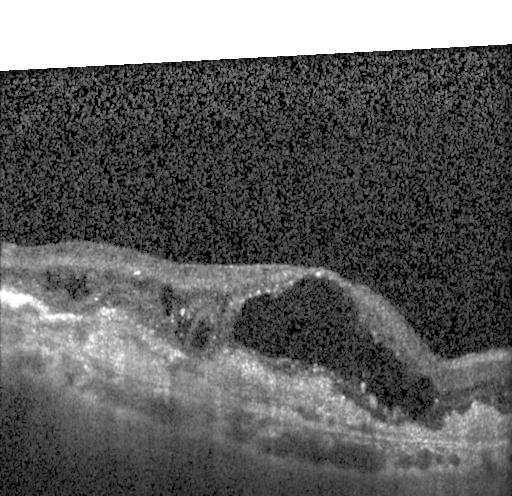

Finding: a choroidal neovascular membrane.